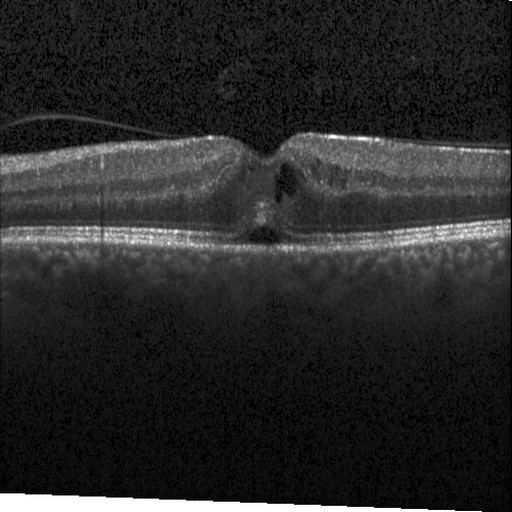

Retinal OCT B-scan · macular scan — Diagnosis: diabetic macular edema.